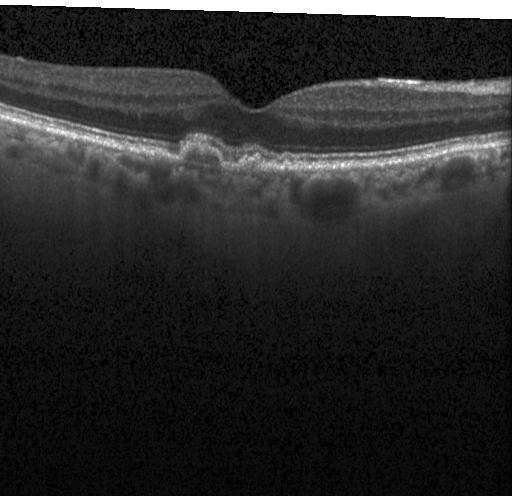
Macular scan · optical coherence tomography scan · instrument: Heidelberg Spectralis
The scan shows a choroidal neovascular membrane.